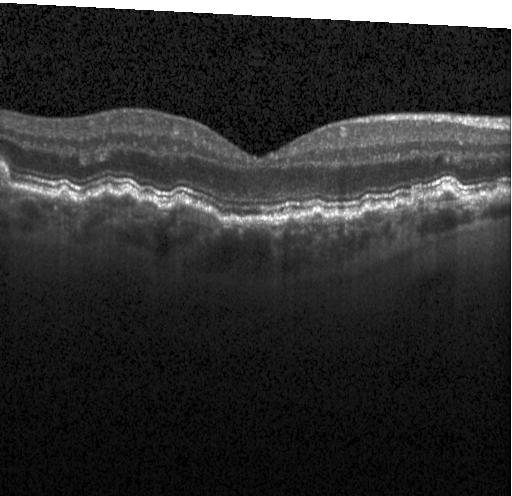
Optical coherence tomography scan; instrument: Heidelberg Spectralis; spectral-domain optical coherence tomography; macular scan — This B-scan demonstrates drusen.